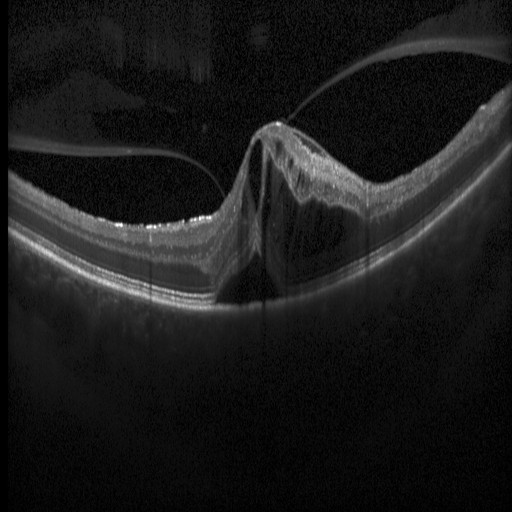
Optical coherence tomography B-scan · centered on the fovea.
The scan shows diabetic macular edema (DME).